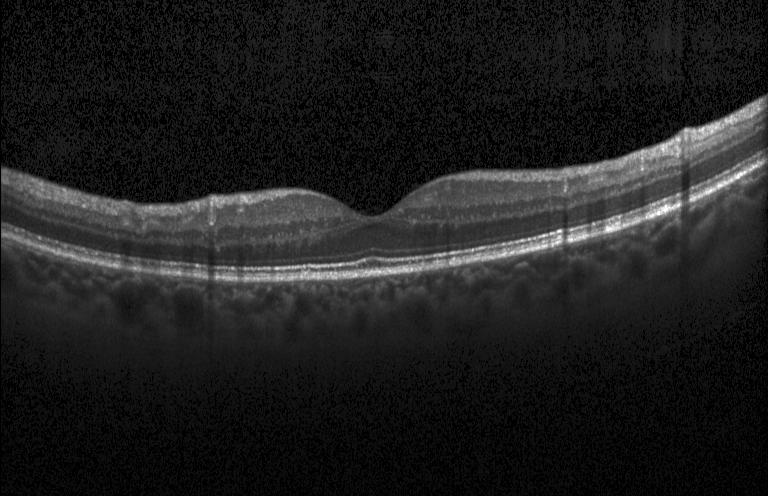
Macular OCT demonstrating neither CNV, DME, nor drusen.